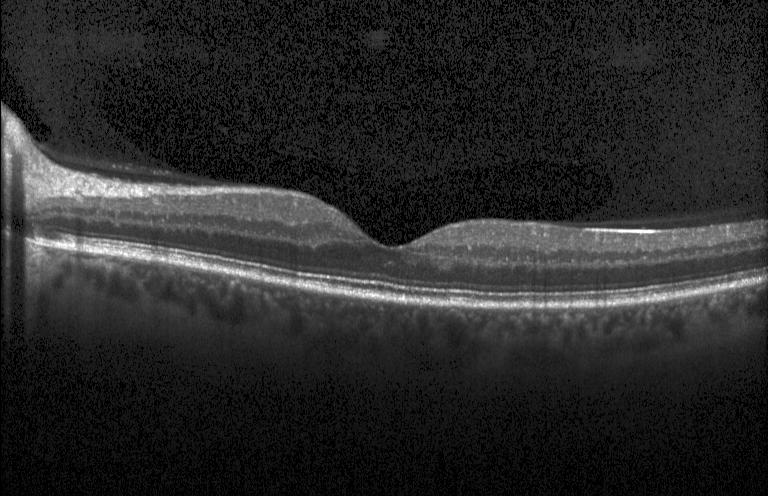 Spectral-domain OCT. Optical coherence tomography B-scan — This B-scan demonstrates no evidence of CNV, DME, or drusen.